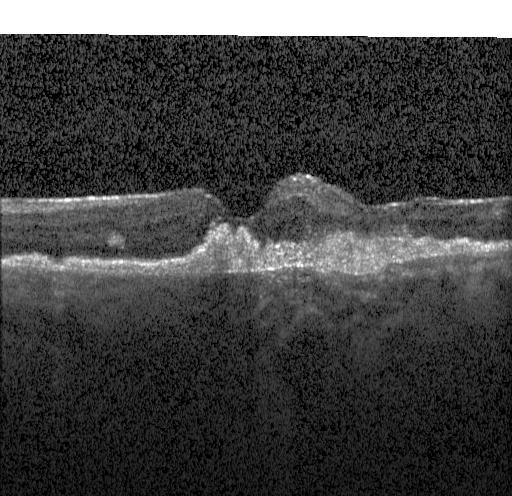
This B-scan demonstrates a choroidal neovascular membrane.